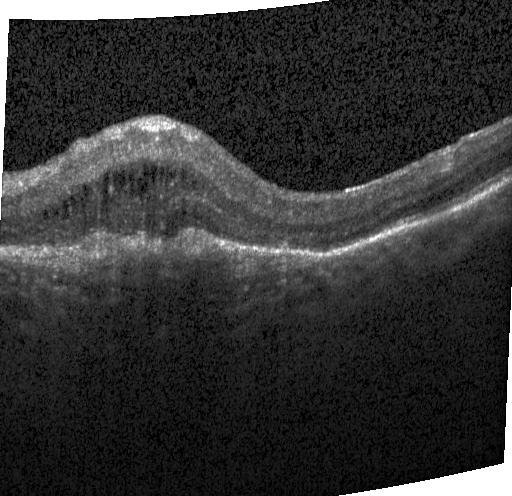

Retinal OCT B-scan · Heidelberg Spectralis · spectral-domain optical coherence tomography · fovea-centered — Impression: a choroidal neovascular membrane.